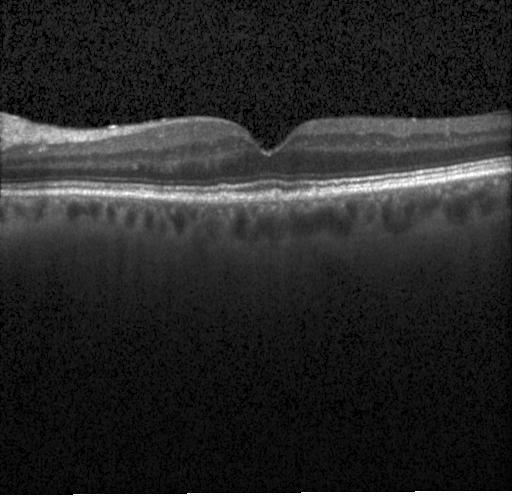
Impression: drusen.